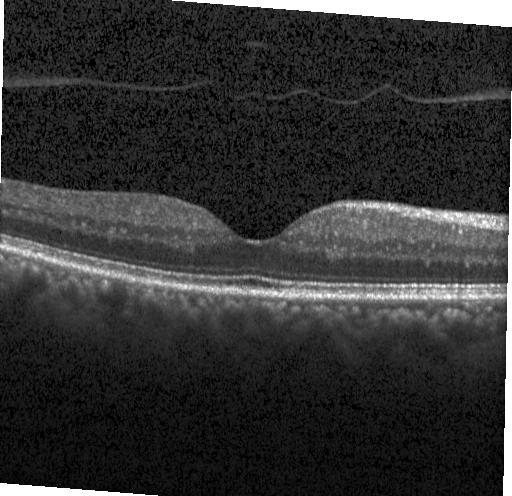
Optical coherence tomography scan, centered on the fovea, spectral-domain OCT.
The scan shows no evidence of choroidal neovascularization, diabetic macular edema, or drusen.